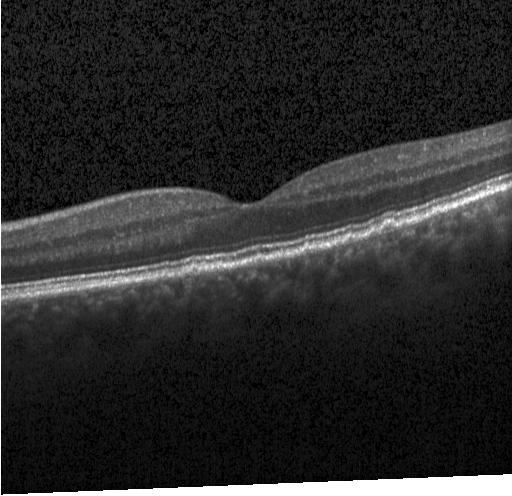

Finding: multiple drusen.